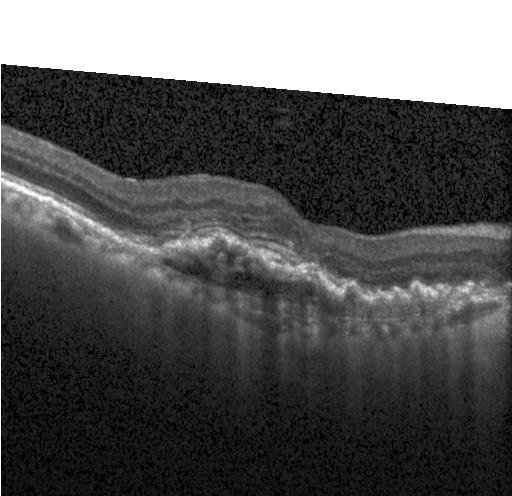

Spectral-domain OCT B-scan: choroidal neovascularization (CNV).